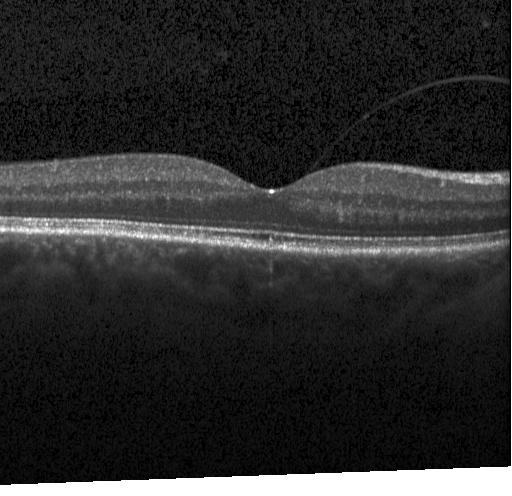 OCT B-scan.
Assessment: no choroidal neovascularization, no diabetic macular edema, and no drusen.